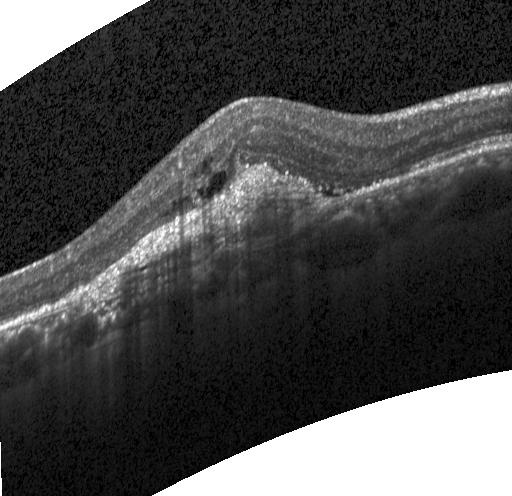 OCT B-scan.
Finding: a choroidal neovascular membrane.